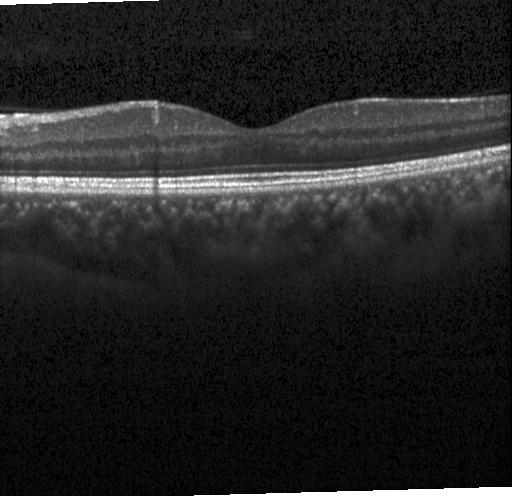
The scan shows no choroidal neovascularization, no diabetic macular edema, and no drusen.